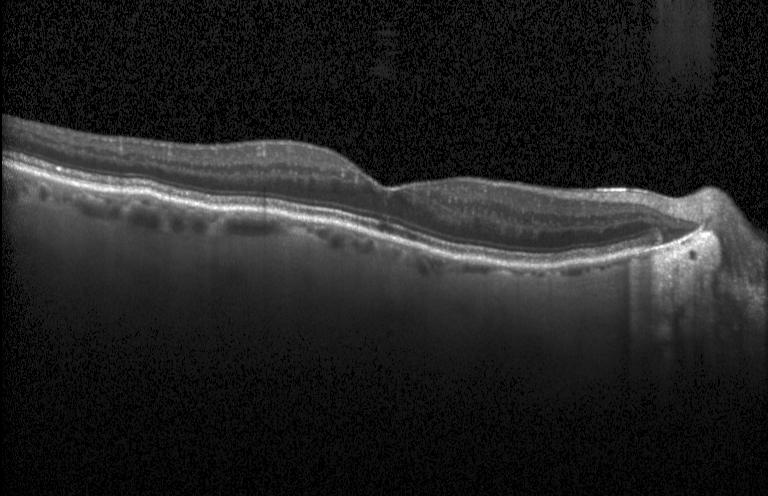
SD-OCT, optical coherence tomography scan. Diagnosis: neither choroidal neovascularization, diabetic macular edema, nor drusen.